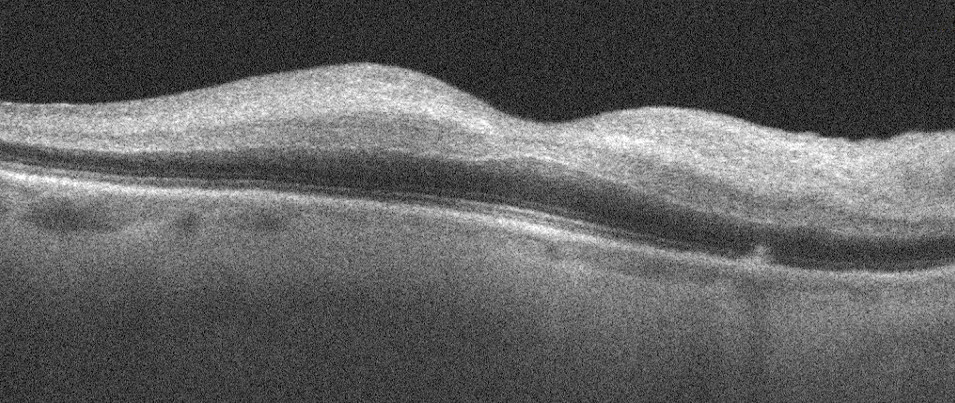 Impression: retinal artery occlusion.